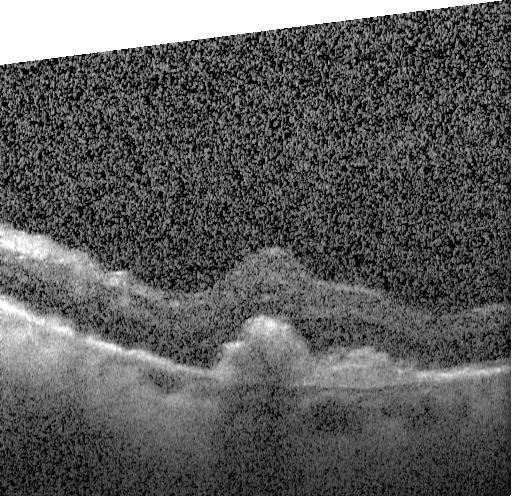

Heidelberg Spectralis · OCT line scan · fovea-centered · spectral-domain optical coherence tomography.
Impression: a choroidal neovascular membrane.